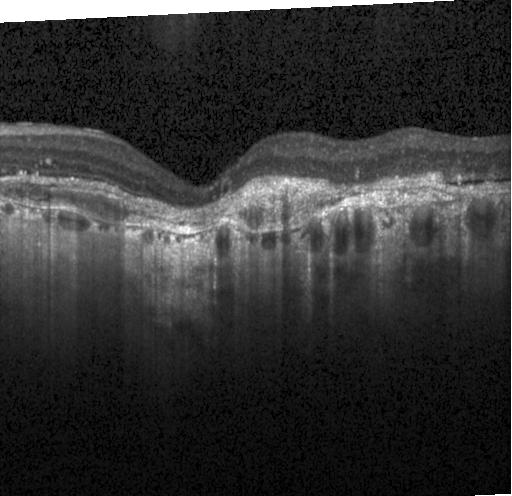
Spectral-domain optical coherence tomography · optical coherence tomography B-scan · through the macula.
Macular OCT: choroidal neovascularization (CNV).